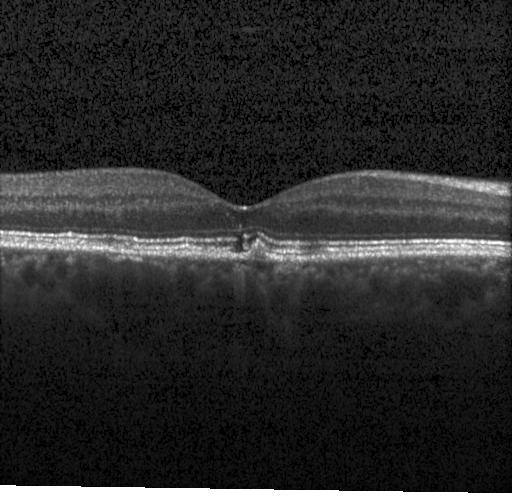

Macular OCT demonstrating CNV.